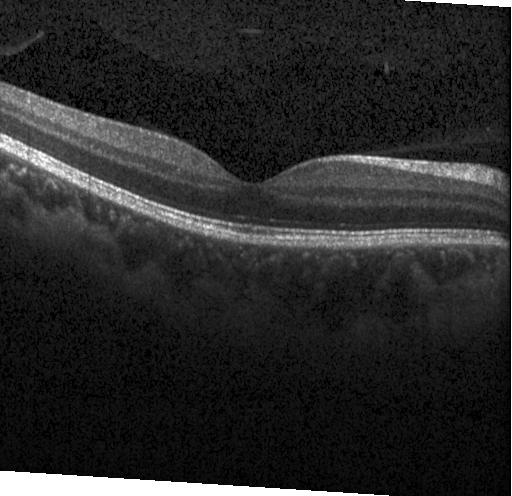 Macular OCT demonstrating neither choroidal neovascularization, diabetic macular edema, nor drusen.